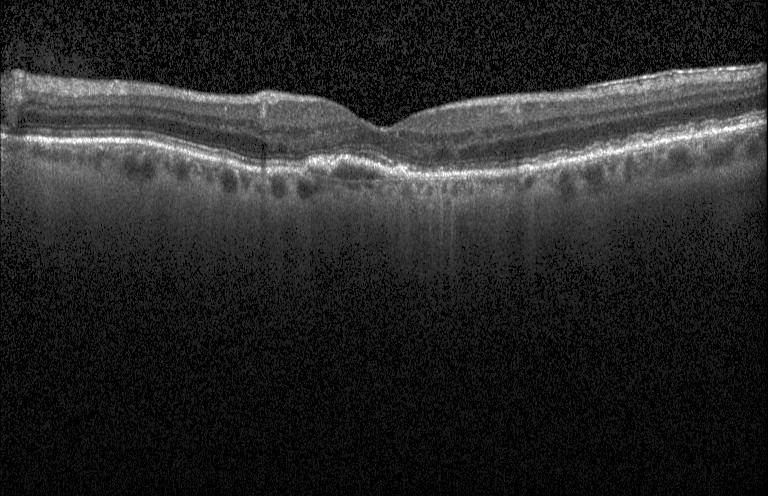
The scan shows choroidal neovascularization (CNV).